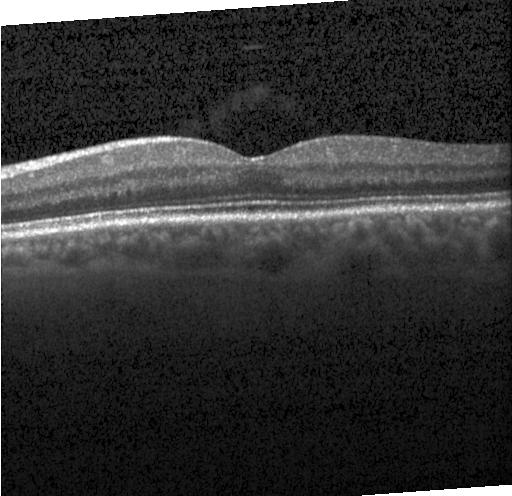 OCT line scan. No choroidal neovascularization, no diabetic macular edema, and no drusen.